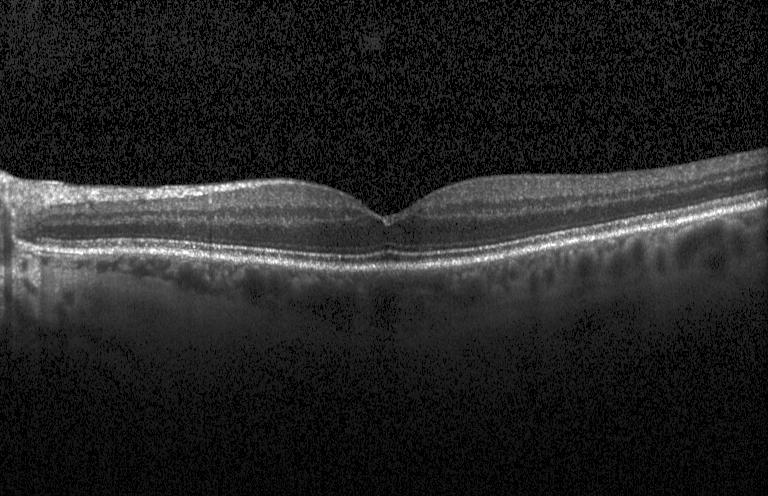

Optical coherence tomography scan; acquired on a Heidelberg Spectralis. Finding: no evidence of choroidal neovascularization, diabetic macular edema, or drusen.